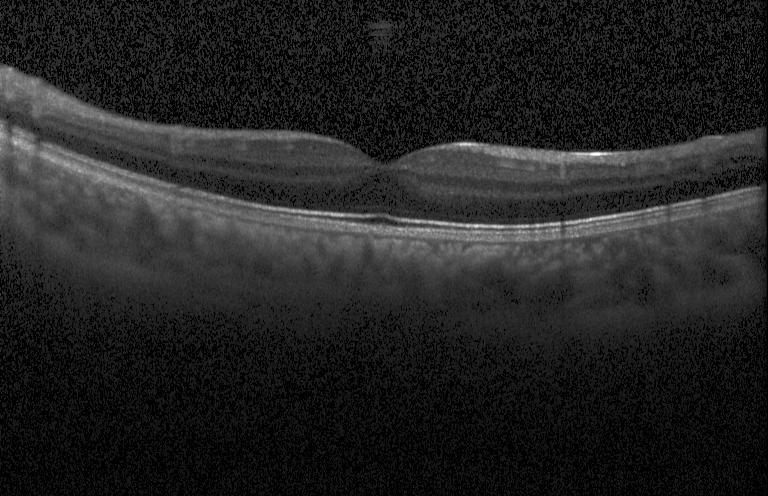 Dx: neither choroidal neovascularization, diabetic macular edema, nor drusen.